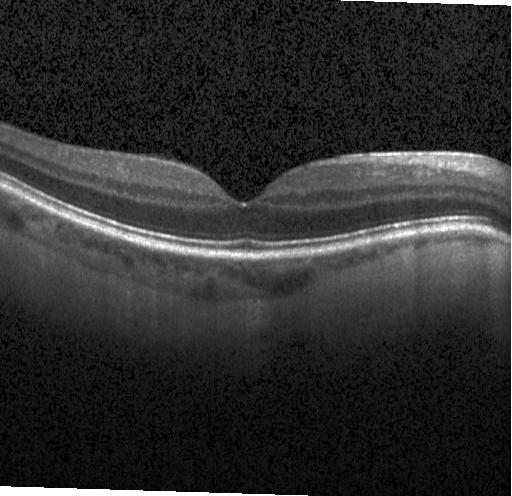

Heidelberg Spectralis. Spectral-domain optical coherence tomography. Centered on the fovea. OCT B-scan. Assessment: no CNV, DME, or drusen.